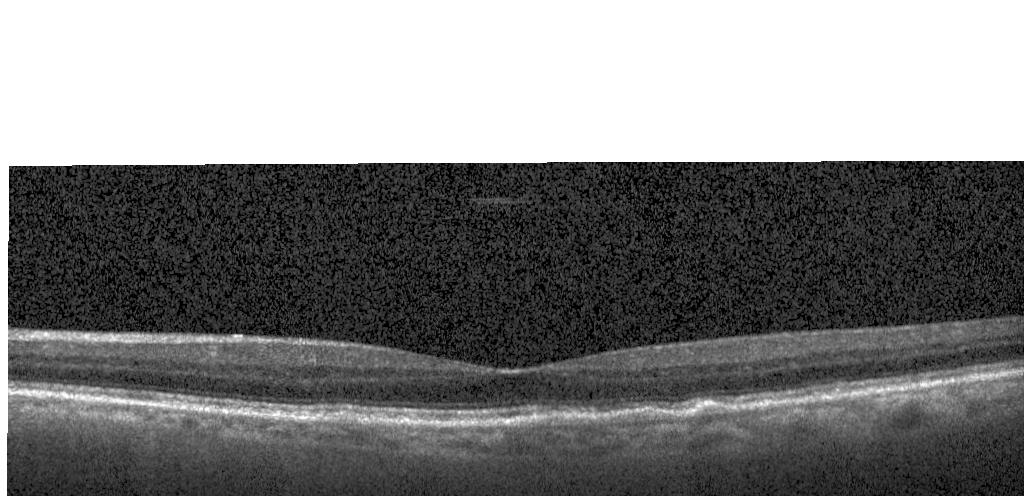

OCT line scan, Heidelberg Spectralis OCT system — Impression: drusen.